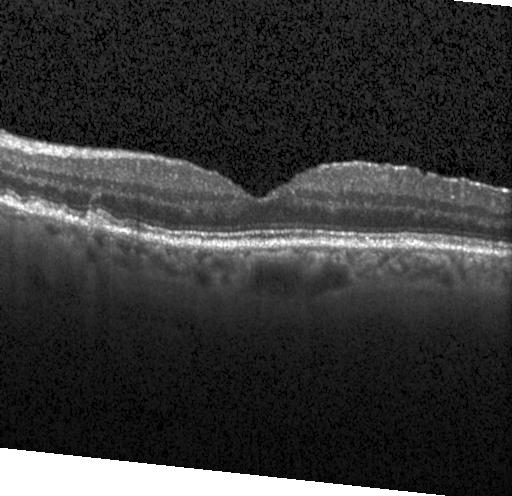

The scan shows multiple drusen.